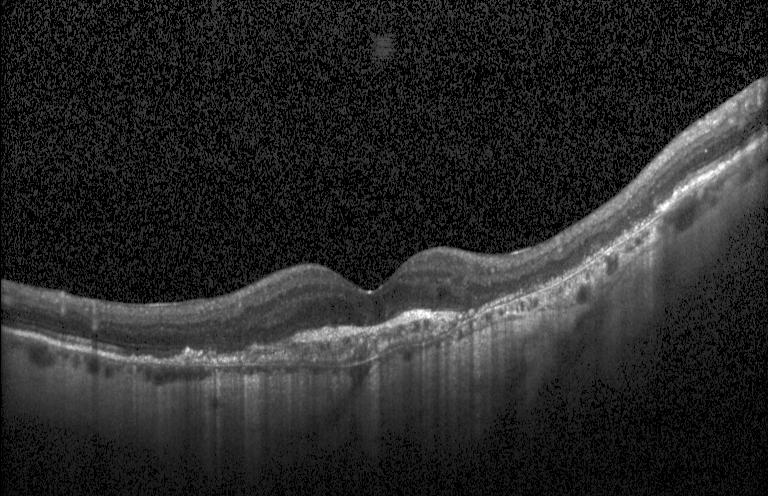

Macular OCT demonstrating a choroidal neovascular membrane.